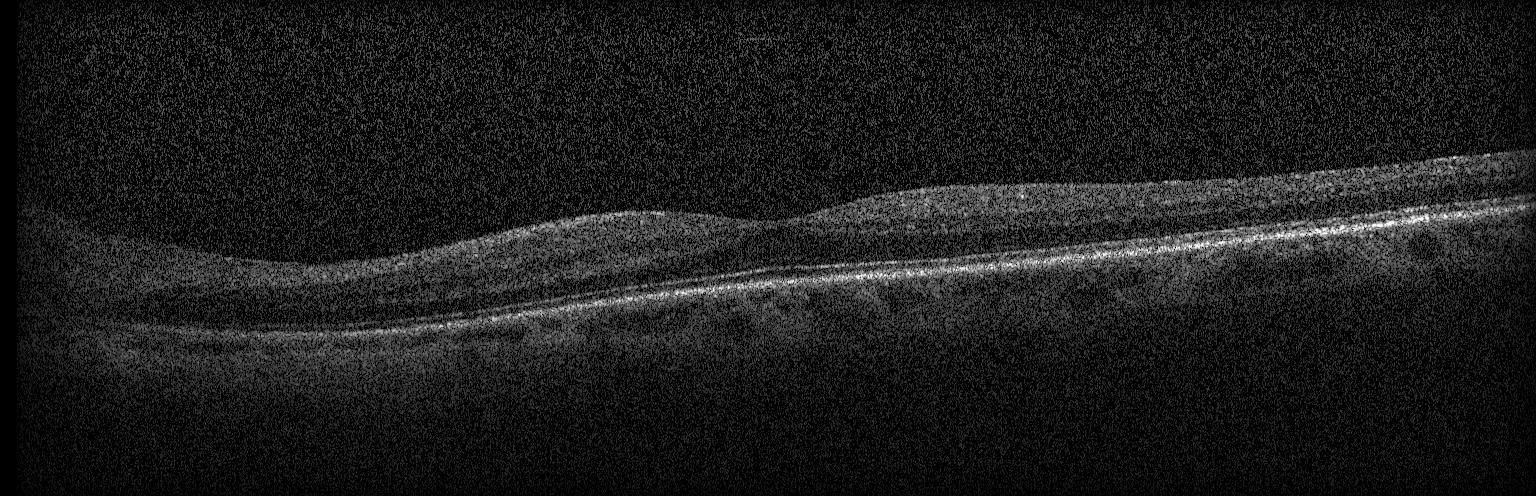
Dx: no CNV, DME, or drusen.